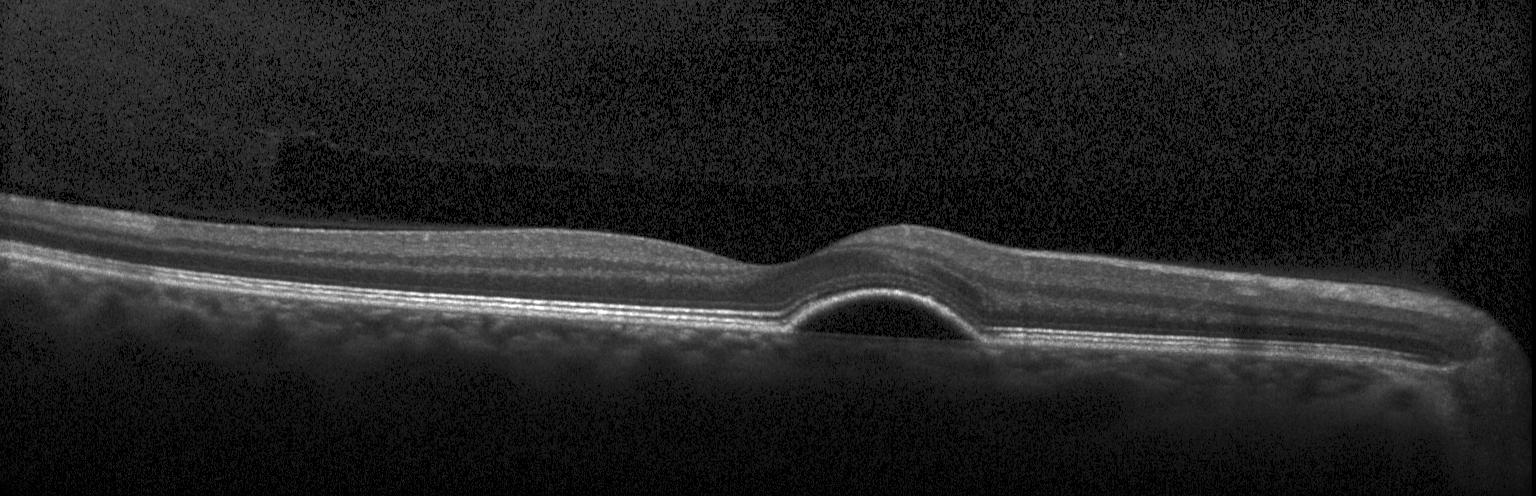 Retinal OCT cross-section — OCT finding: a choroidal neovascular membrane.